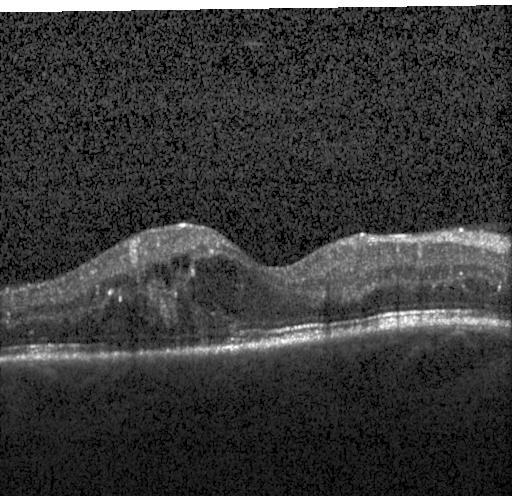
Through the macula; optical coherence tomography B-scan — Diabetic macular edema (DME).